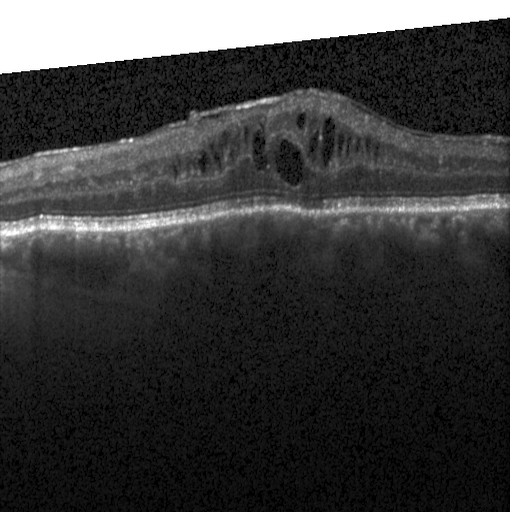 Finding: DME.